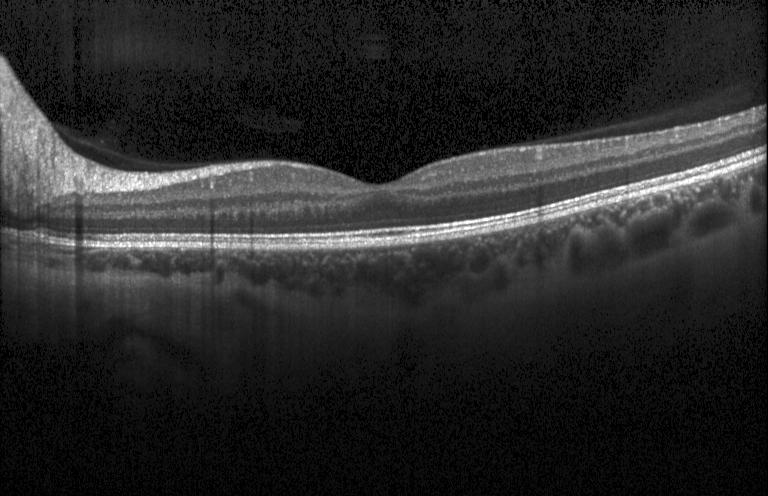

Diagnosis: no choroidal neovascularization, diabetic macular edema, or drusen.